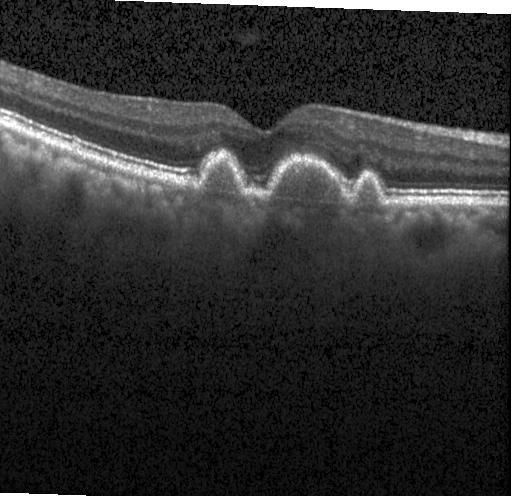
Finding: sub-RPE drusenoid deposits.